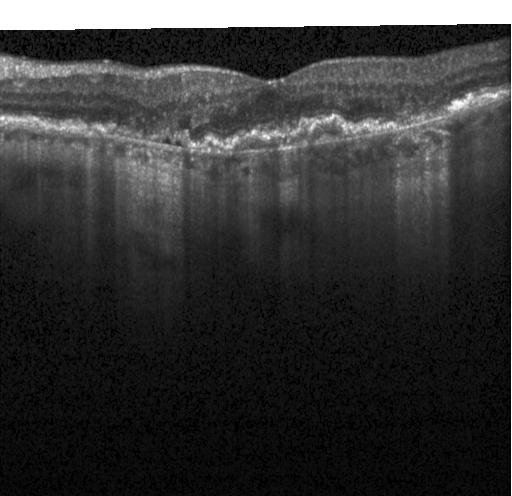
Diagnosis: CNV.